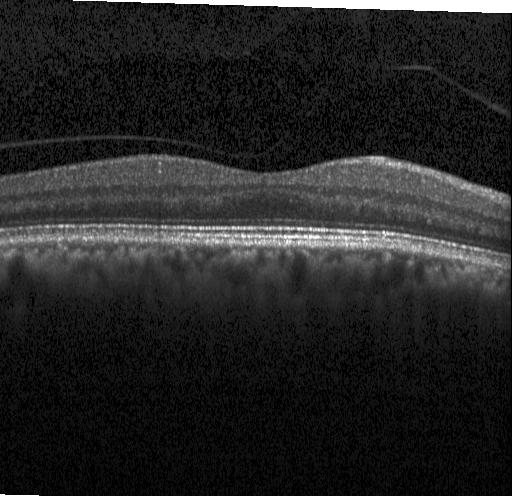
Retinal OCT cross-section
Finding: no evidence of choroidal neovascularization, diabetic macular edema, or drusen.